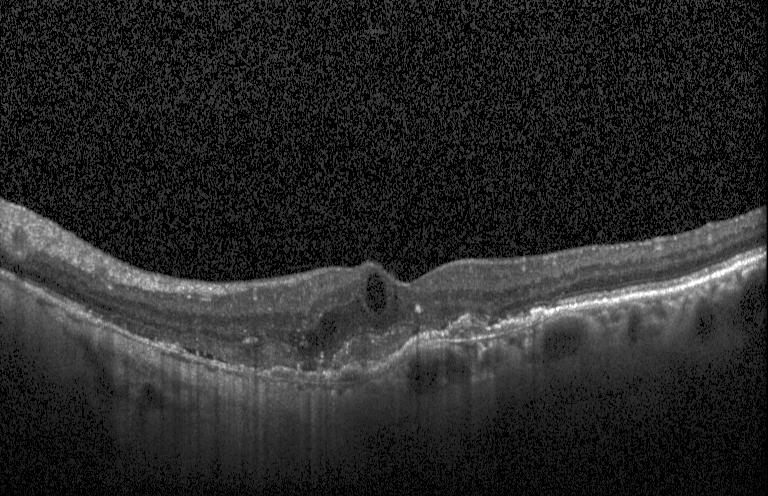

Heidelberg Spectralis OCT system. Optical coherence tomography B-scan. Horizontal scan through the fovea. SD-OCT. Impression: a choroidal neovascular membrane.